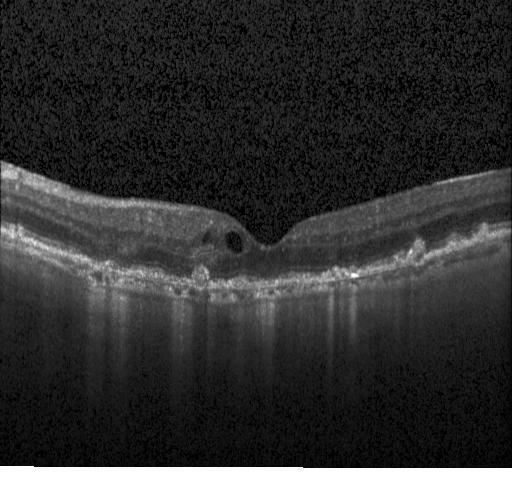 SD-OCT · OCT B-scan
Assessment: a choroidal neovascular membrane.